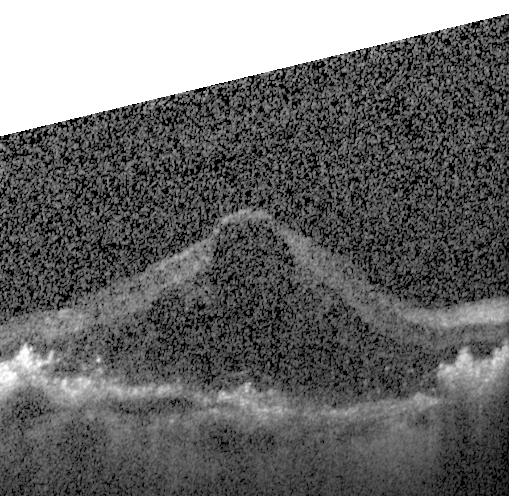 Fovea-centered; retinal OCT B-scan
Dx: choroidal neovascularization.